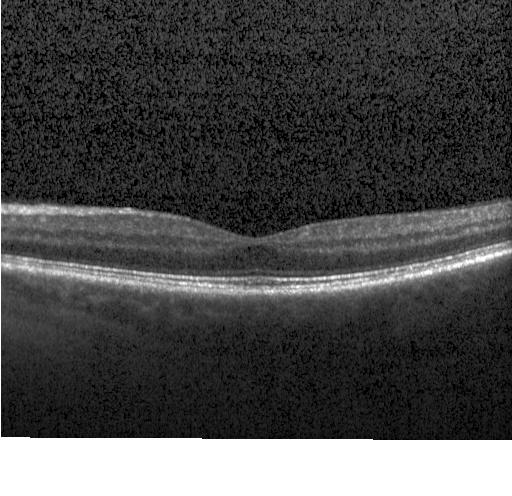
Optical coherence tomography B-scan; spectral-domain OCT; fovea-centered
OCT finding: no evidence of choroidal neovascularization, diabetic macular edema, or drusen.